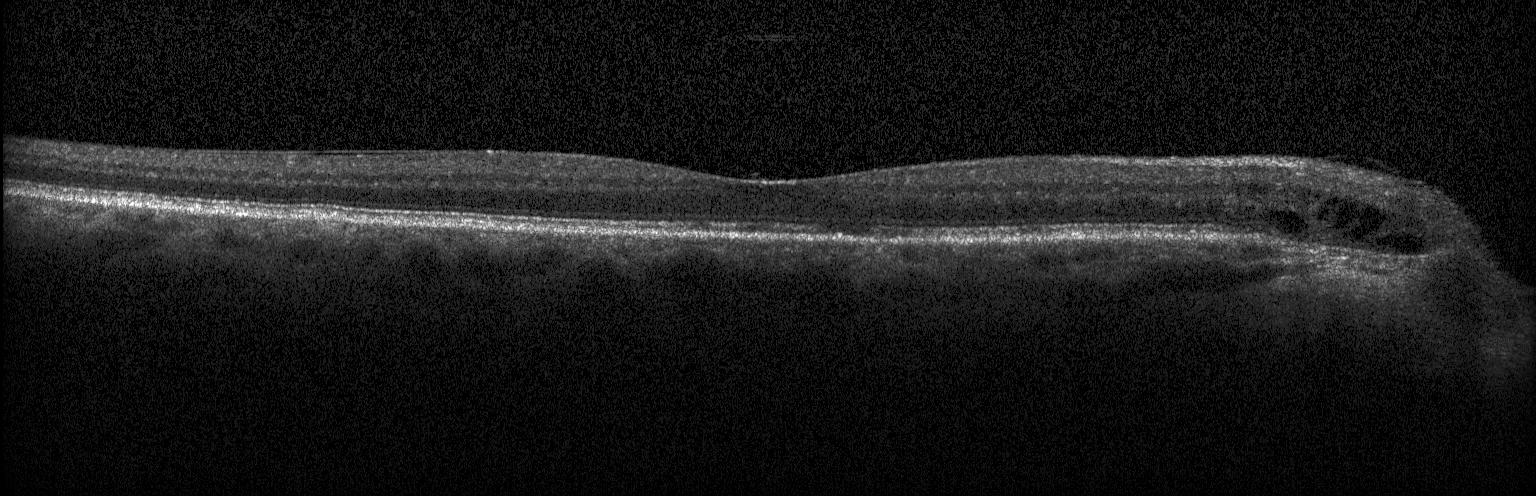
Retinal OCT B-scan, Heidelberg Spectralis OCT system, SD-OCT, horizontal scan through the fovea — Dx: DME.